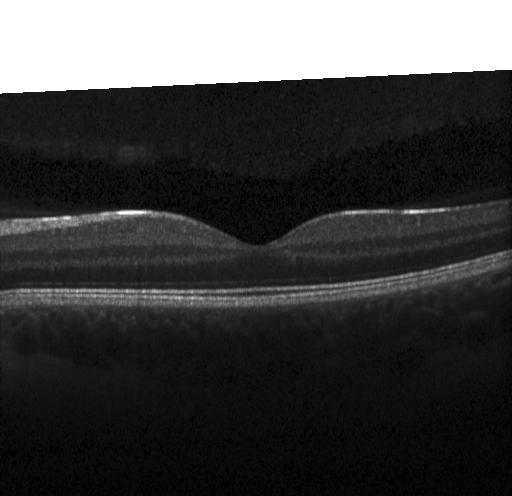 Macular OCT: neither CNV, DME, nor drusen.